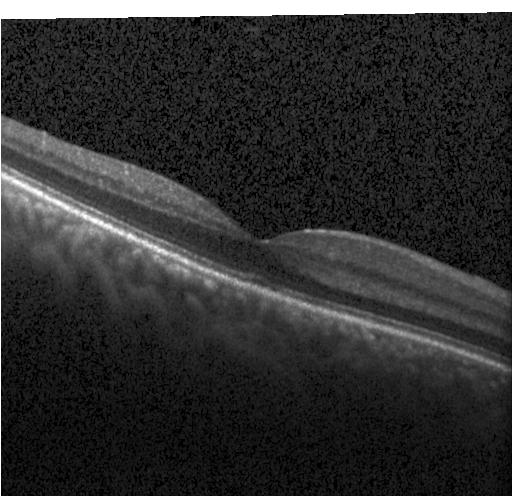
Acquired on a Heidelberg Spectralis; spectral-domain OCT; OCT line scan; through the macula
The scan shows no choroidal neovascularization, diabetic macular edema, or drusen.